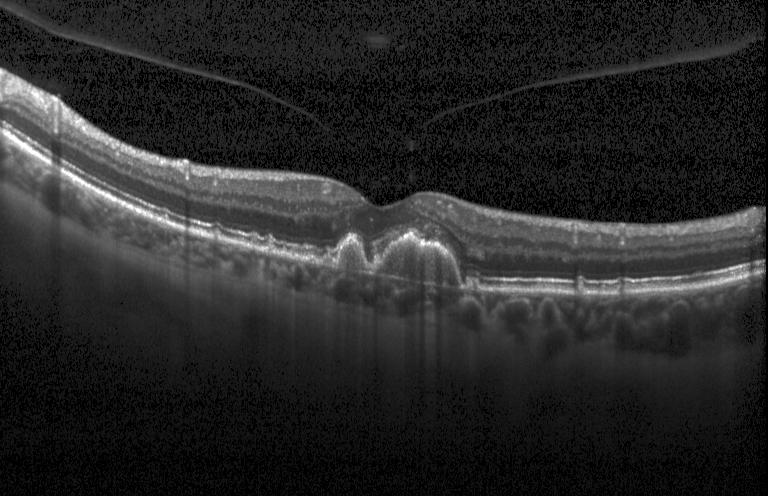

OCT scan showing a choroidal neovascular membrane.